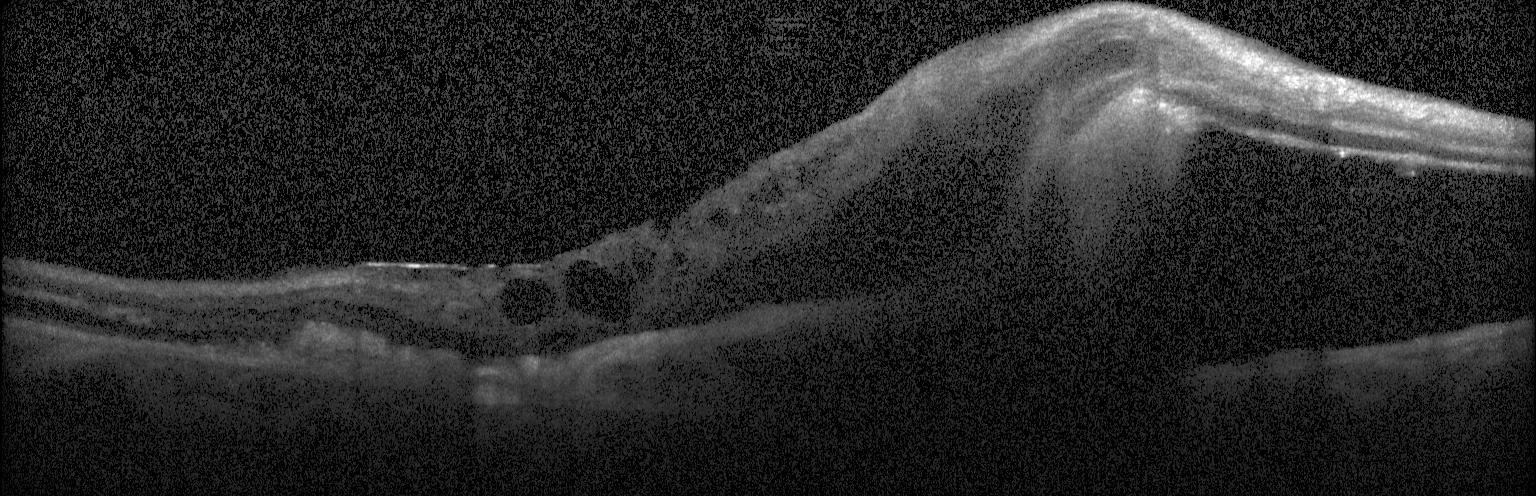
Optical coherence tomography B-scan.
Choroidal neovascularization.